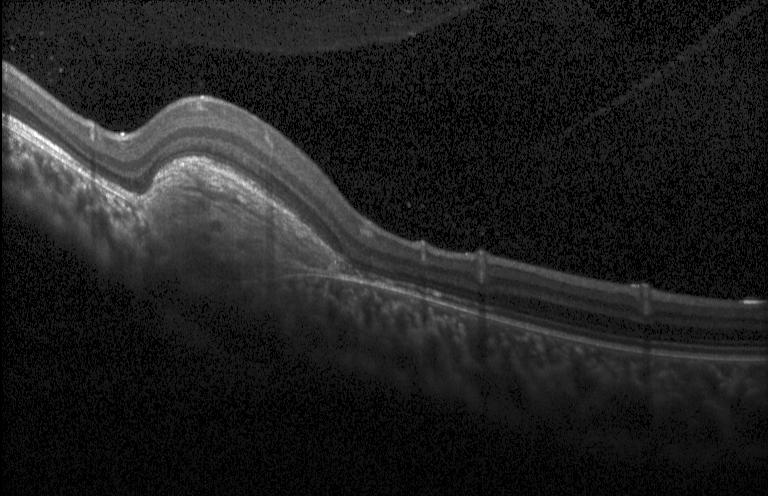

Macular OCT: choroidal neovascularization (CNV).